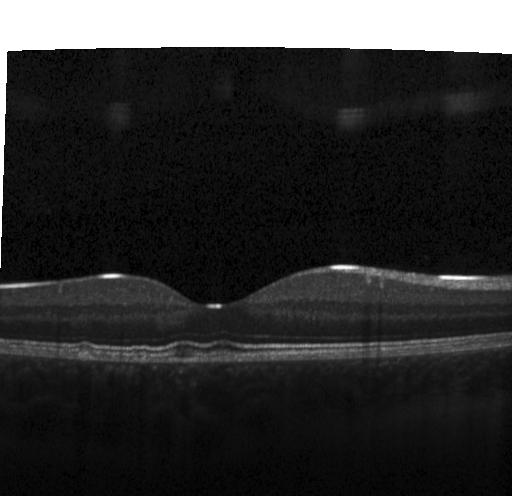
Finding: sub-RPE drusenoid deposits.